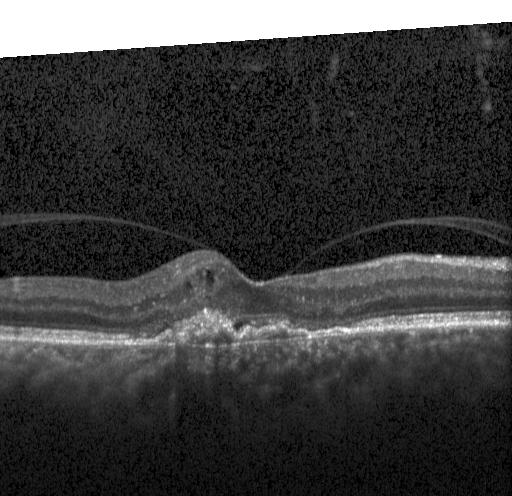

Optical coherence tomography B-scan. Centered on the fovea. Diagnosis: choroidal neovascularization (CNV).